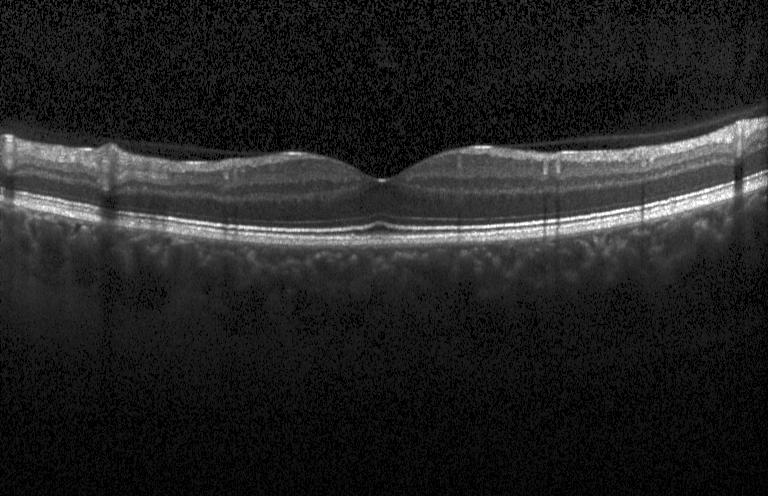 Spectral-domain optical coherence tomography. OCT B-scan
Impression: no choroidal neovascularization, diabetic macular edema, or drusen.